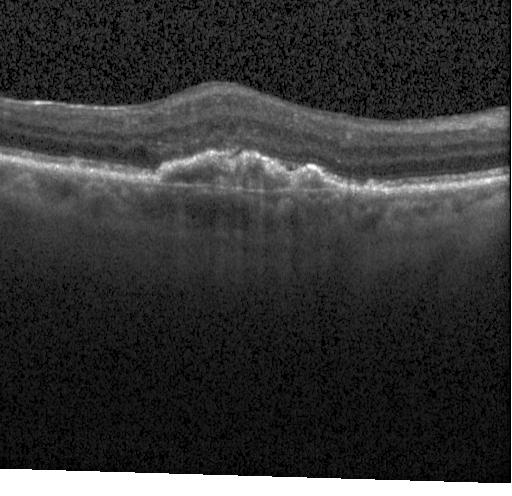

This B-scan demonstrates choroidal neovascularization (CNV).